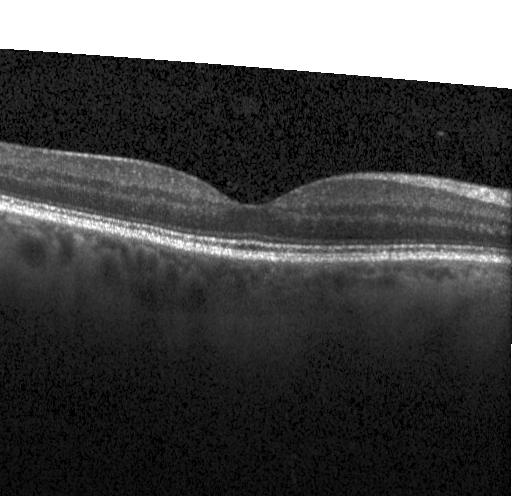 OCT B-scan showing no CNV, no DME, and no drusen.